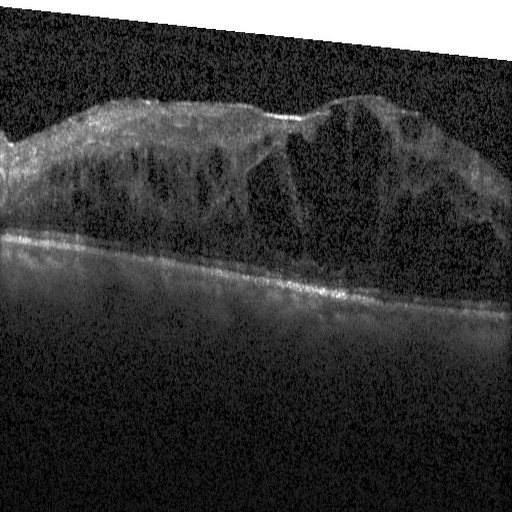
Horizontal scan through the fovea. Retinal OCT cross-section. Spectral-domain optical coherence tomography
Diagnosis: diabetic macular edema.